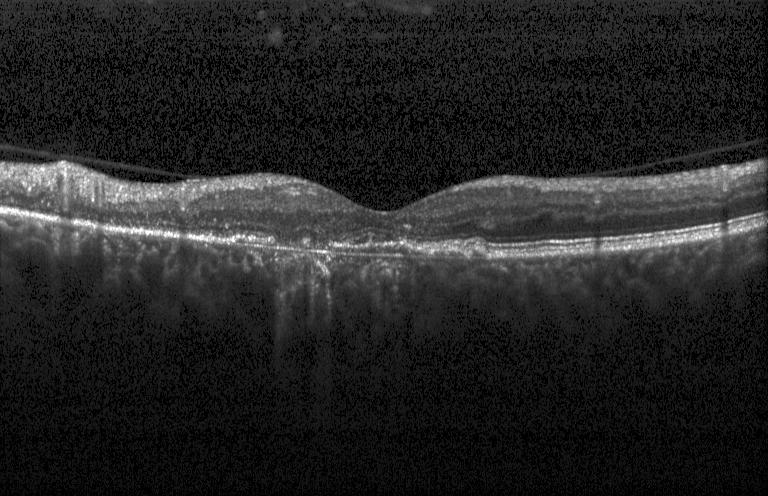

Impression: a choroidal neovascular membrane.